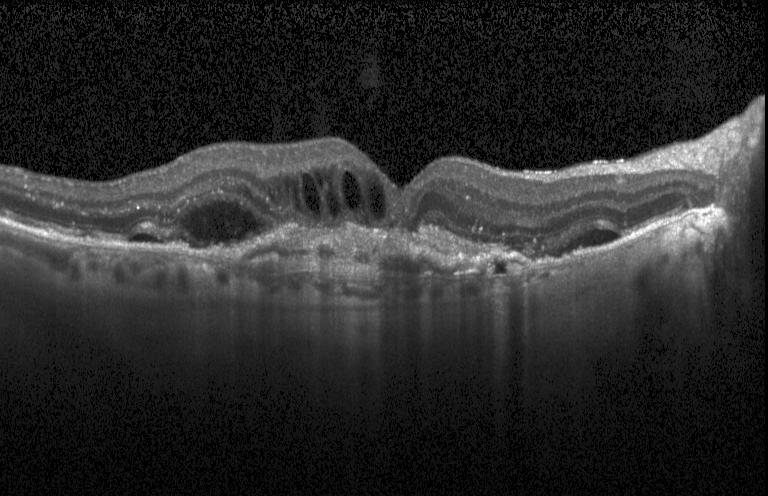
Macular scan. Instrument: Heidelberg Spectralis. Retinal OCT cross-section. Spectral-domain optical coherence tomography.
This B-scan demonstrates choroidal neovascularization (CNV).